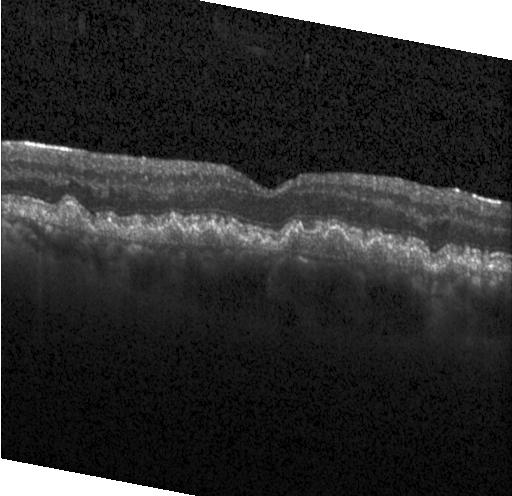

Diagnosis: CNV.